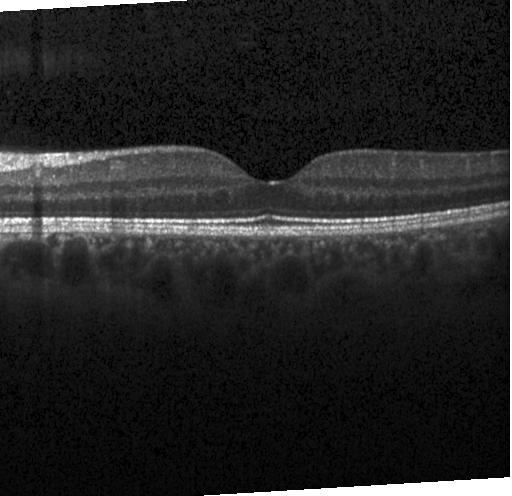

Optical coherence tomography B-scan · horizontal scan through the fovea
Finding: no choroidal neovascularization, no diabetic macular edema, and no drusen.